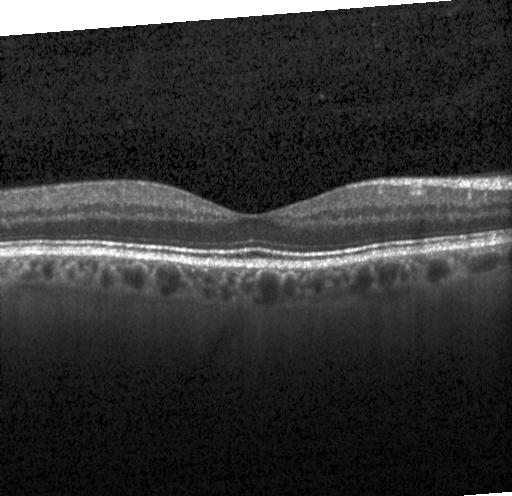 Centered on the fovea · Heidelberg Spectralis · SD-OCT · retinal OCT cross-section. Diagnosis: no evidence of choroidal neovascularization, diabetic macular edema, or drusen.